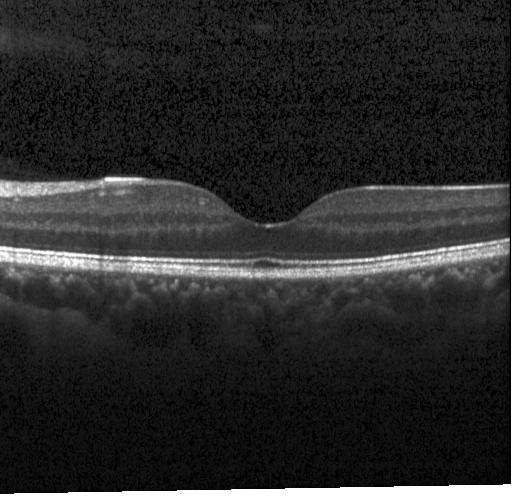
Macular OCT: no evidence of choroidal neovascularization, diabetic macular edema, or drusen.